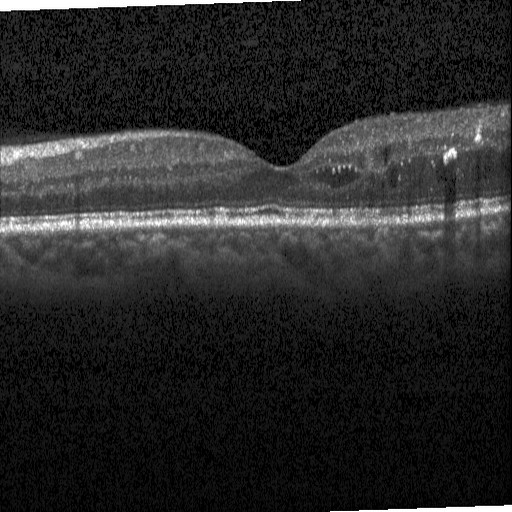
Retinal OCT cross-section.
Finding: diabetic macular edema (DME).